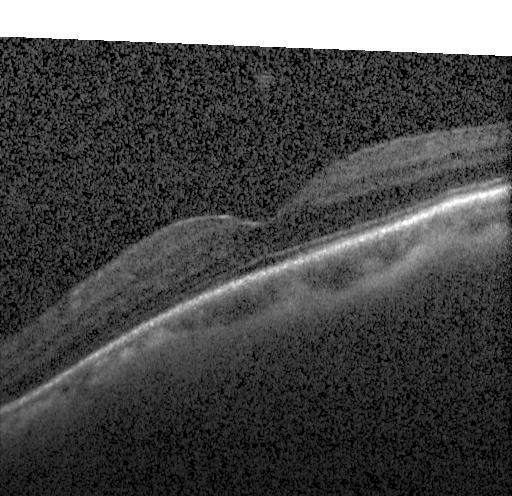

OCT finding: no evidence of choroidal neovascularization, diabetic macular edema, or drusen.